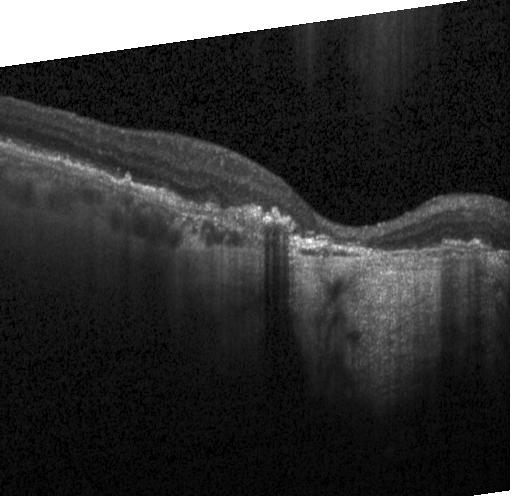

OCT scan showing a choroidal neovascular membrane.